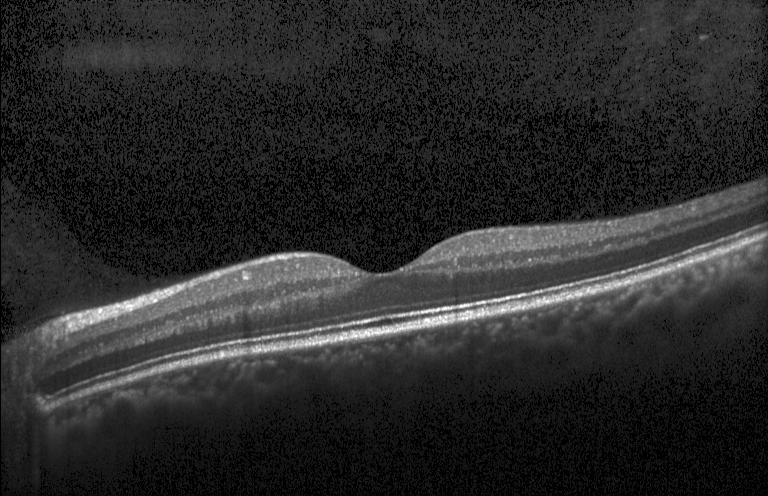

Retinal OCT cross-section. Diagnosis: no evidence of choroidal neovascularization, diabetic macular edema, or drusen.